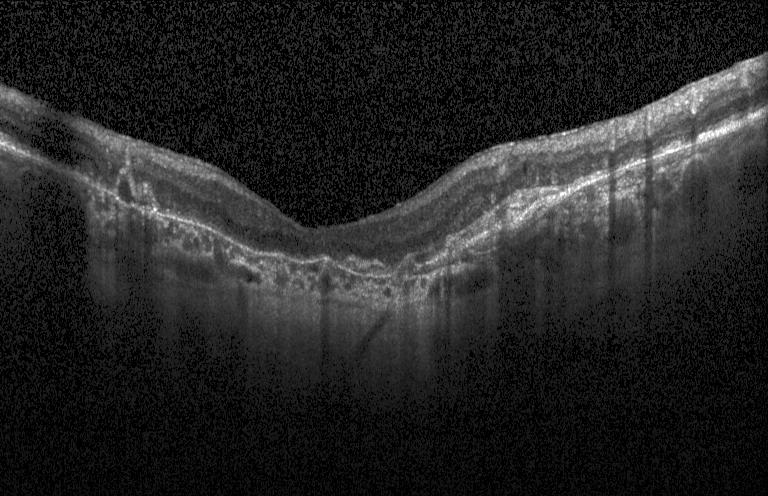

Optical coherence tomography B-scan. Assessment: a choroidal neovascular membrane.